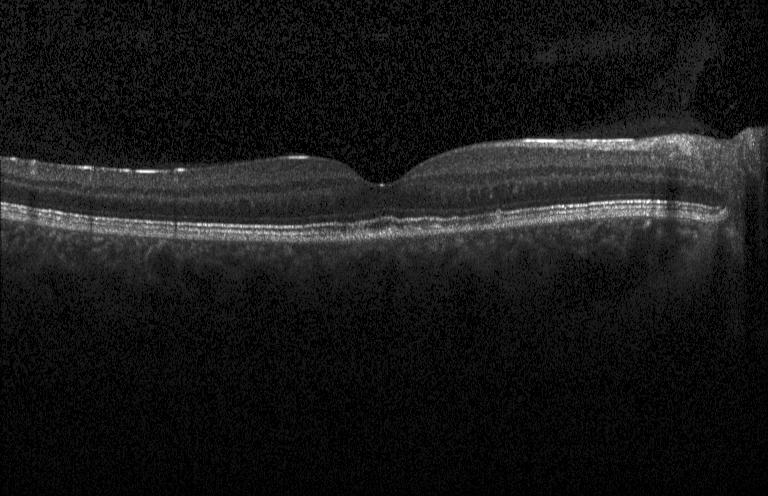 OCT finding: sub-RPE drusenoid deposits.